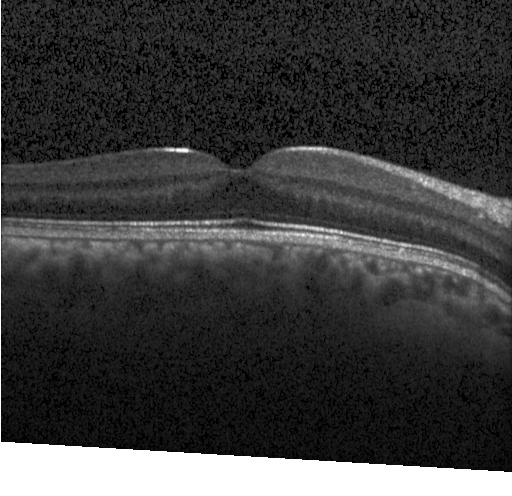 Instrument: Heidelberg Spectralis. Centered on the fovea. SD-OCT. Retinal OCT B-scan. OCT finding: no evidence of choroidal neovascularization, diabetic macular edema, or drusen.